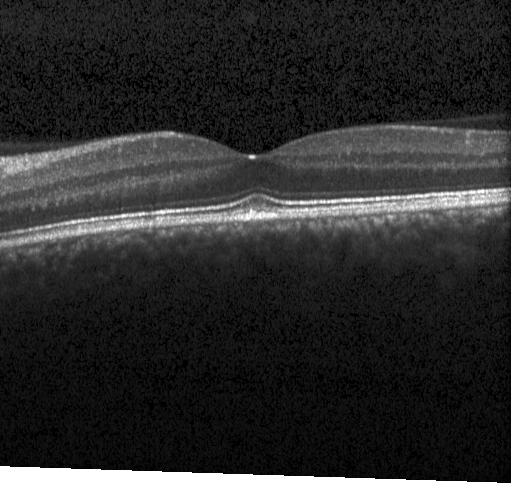

Retinal OCT B-scan · SD-OCT.
Impression: neither choroidal neovascularization, diabetic macular edema, nor drusen.